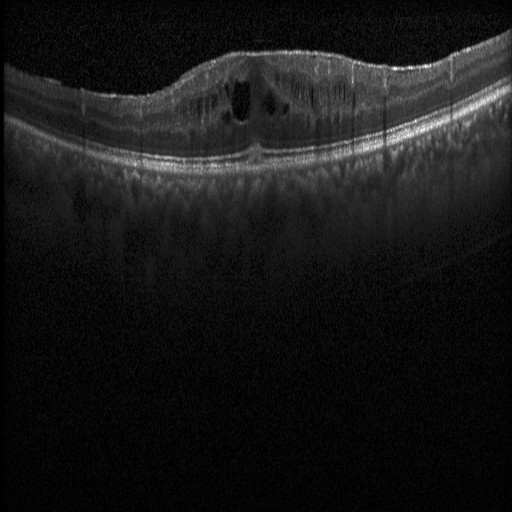 Impression: diabetic macular edema.